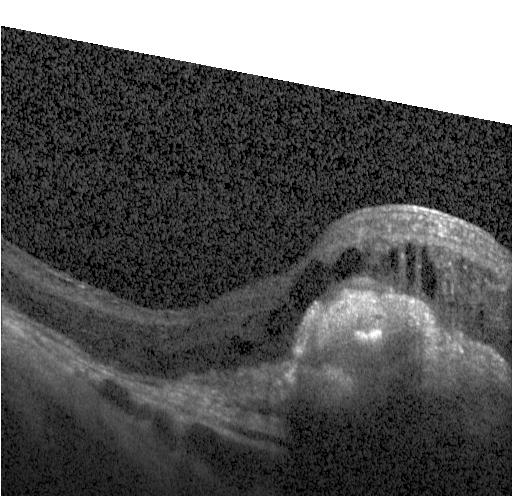
Retinal OCT cross-section — Finding: a choroidal neovascular membrane.